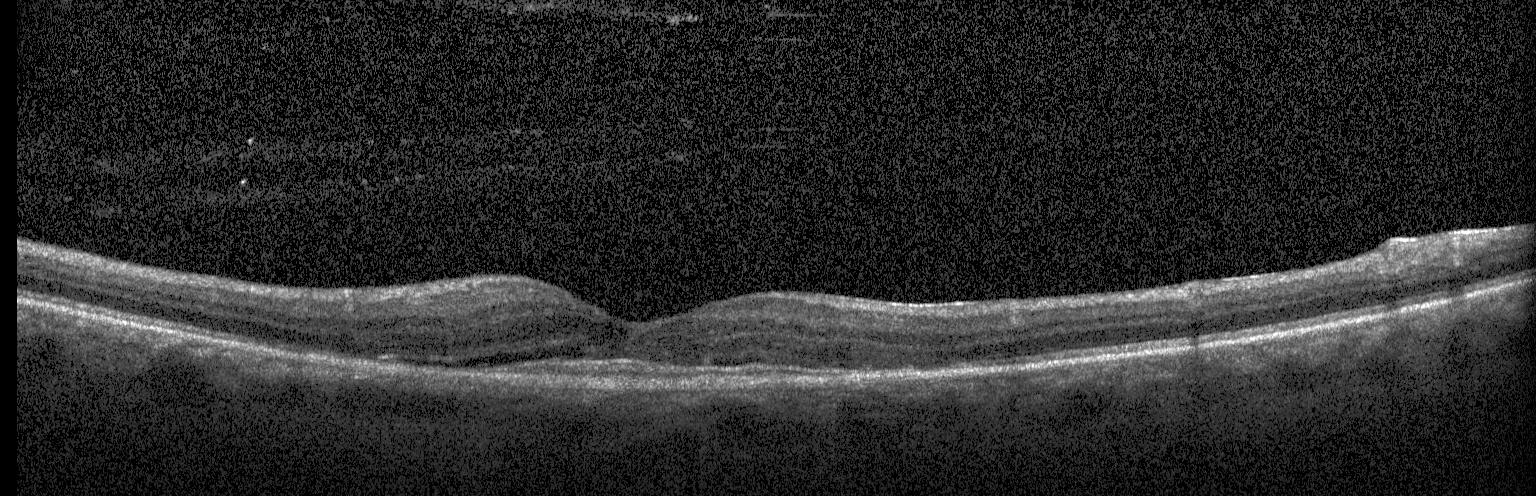
Horizontal scan through the fovea; retinal OCT cross-section.
The scan shows a choroidal neovascular membrane.